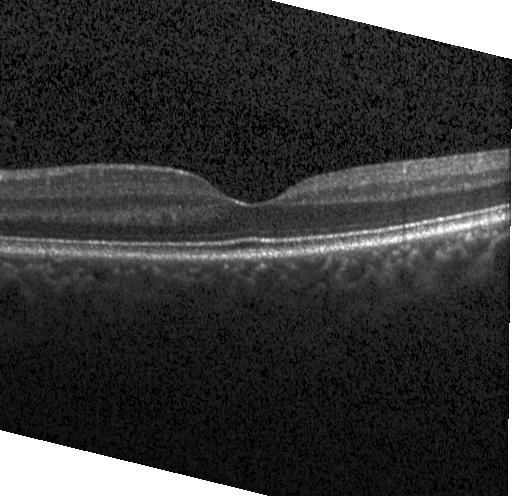

OCT line scan; Heidelberg Spectralis OCT system
Diagnosis: no choroidal neovascularization, no diabetic macular edema, and no drusen.